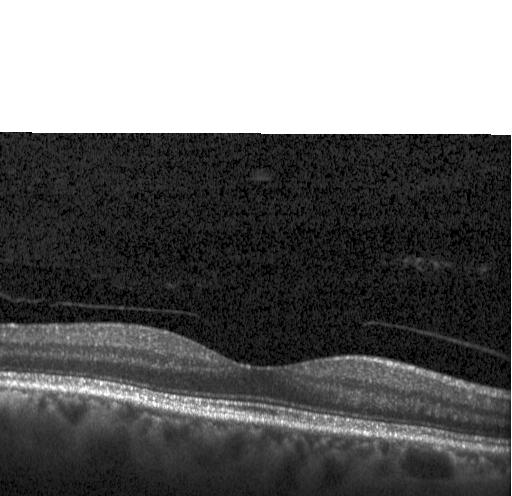
Retinal OCT cross-section.
Diagnosis: no choroidal neovascularization, no diabetic macular edema, and no drusen.